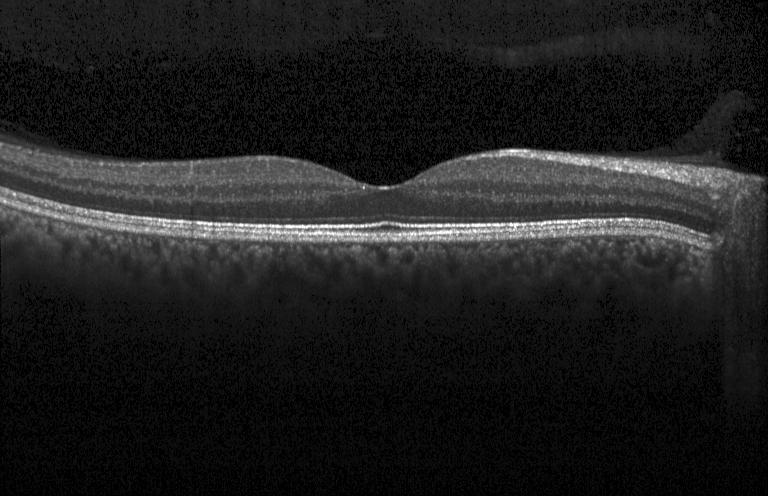 OCT scan showing no choroidal neovascularization, no diabetic macular edema, and no drusen.